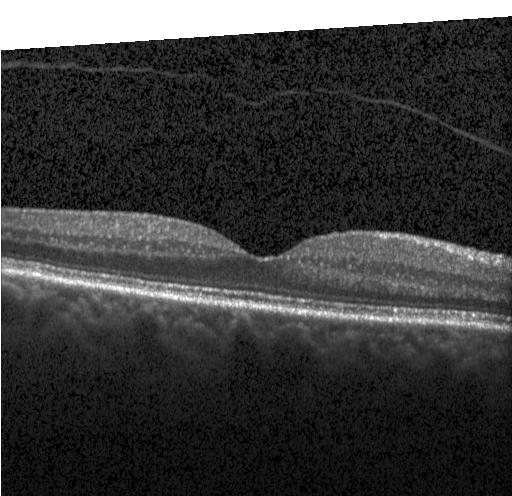
Spectral-domain optical coherence tomography, centered on the fovea, instrument: Heidelberg Spectralis, OCT line scan — The scan shows neither choroidal neovascularization, diabetic macular edema, nor drusen.